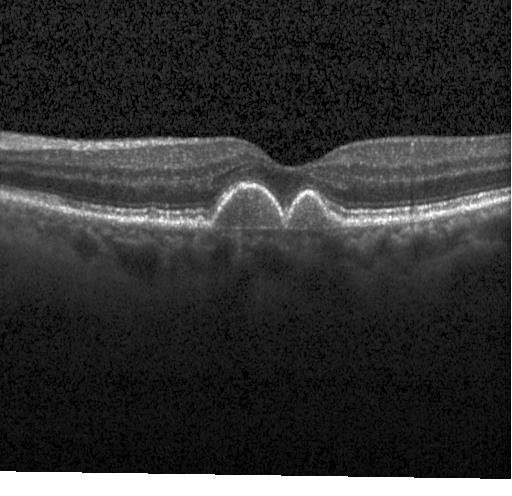
Retinal OCT B-scan — Sub-RPE drusenoid deposits.